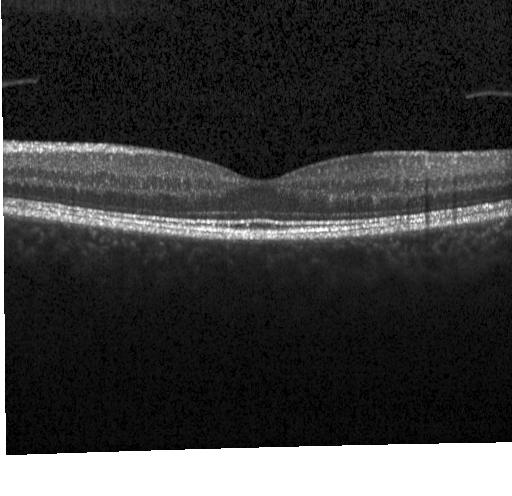 Retinal OCT cross-section showing no choroidal neovascularization, no diabetic macular edema, and no drusen.